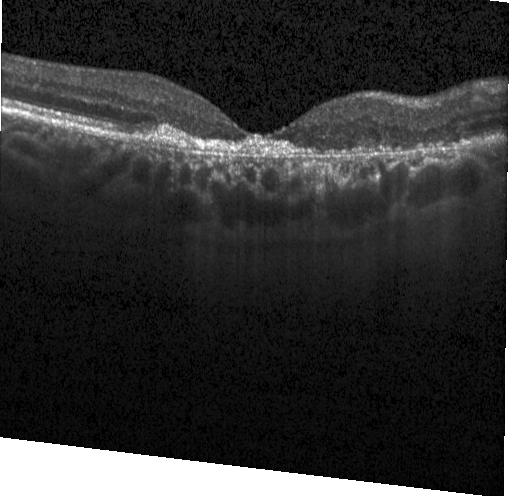 Optical coherence tomography B-scan · through the macula · SD-OCT · acquired on a Heidelberg Spectralis — Dx: a choroidal neovascular membrane.